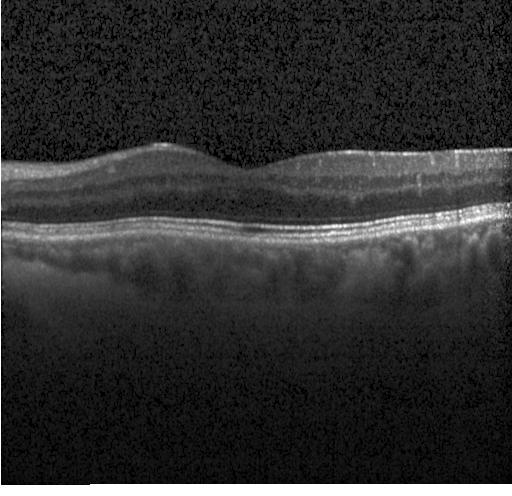

Fovea-centered, spectral-domain OCT, Heidelberg Spectralis OCT system, retinal OCT B-scan.
Macular OCT: neither choroidal neovascularization, diabetic macular edema, nor drusen.